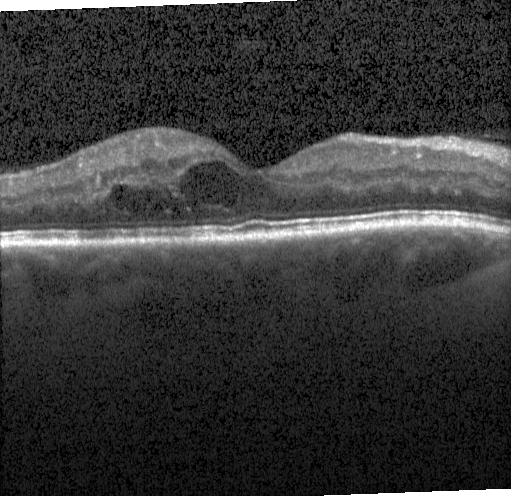

OCT finding: diabetic macular edema.